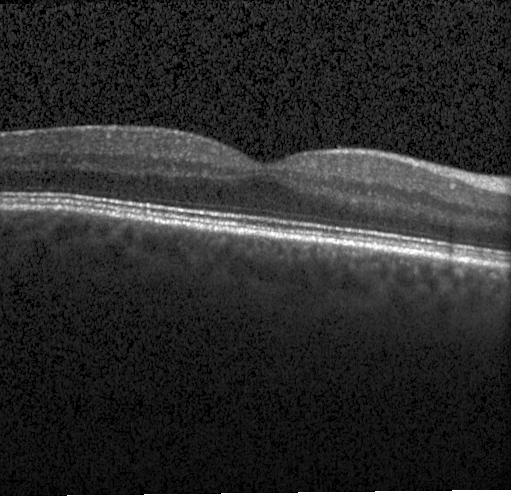

OCT finding: no CNV, DME, or drusen.